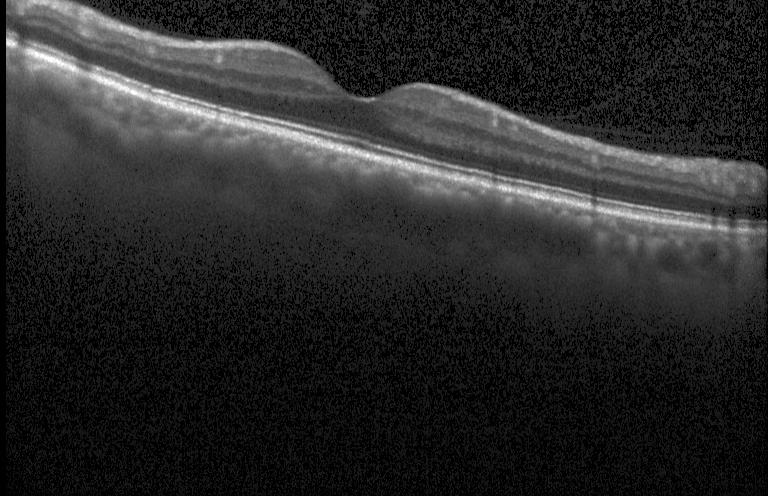

Optical coherence tomography scan. Acquired on a Heidelberg Spectralis. Through the macula. Spectral-domain optical coherence tomography.
No CNV, DME, or drusen.